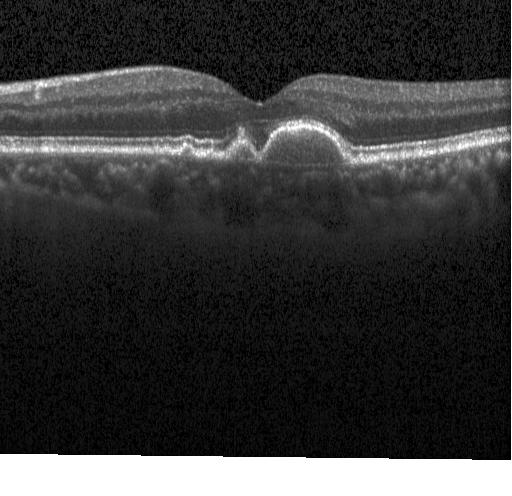

Optical coherence tomography B-scan, through the macula, SD-OCT, acquired on a Heidelberg Spectralis.
Diagnosis: sub-RPE drusenoid deposits.